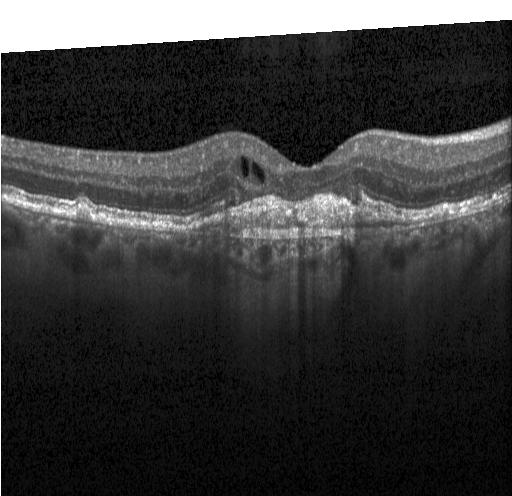
OCT line scan. Horizontal scan through the fovea. Instrument: Heidelberg Spectralis. SD-OCT
Finding: choroidal neovascularization (CNV).